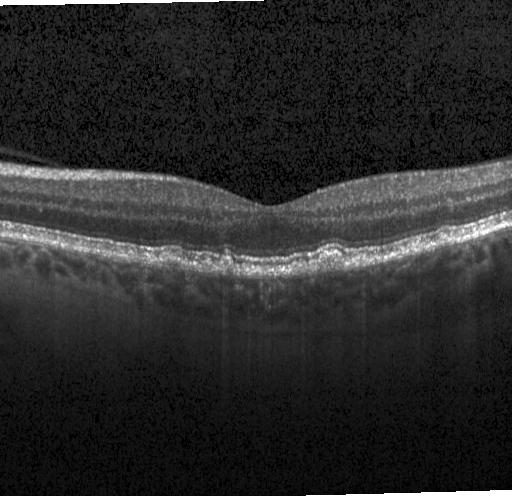

Diagnosis: multiple drusen.